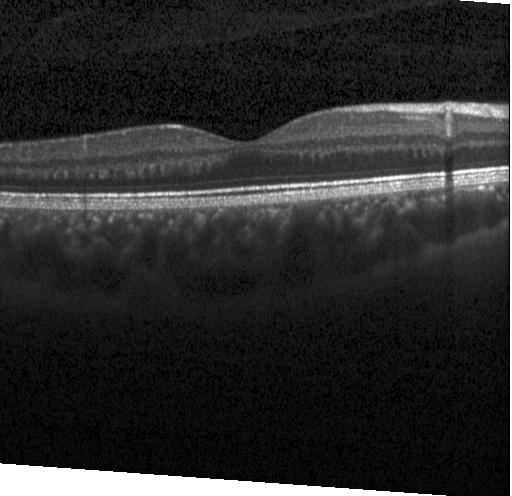

Optical coherence tomography B-scan, fovea-centered. Assessment: no choroidal neovascularization, diabetic macular edema, or drusen.